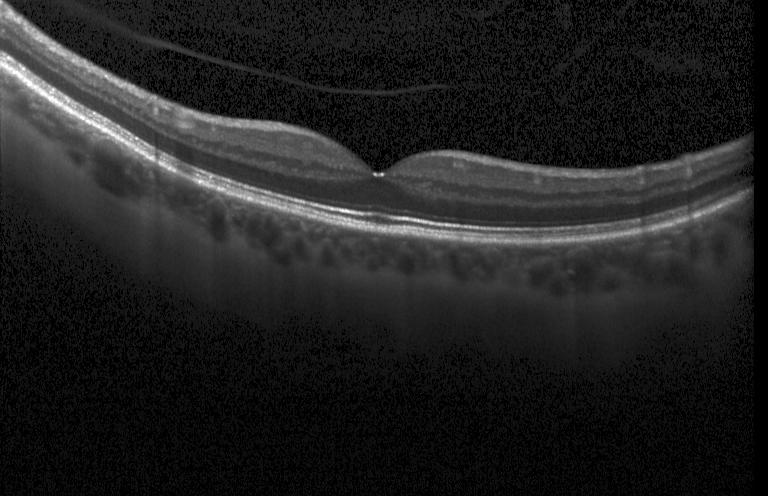
OCT line scan. Acquired on a Heidelberg Spectralis. Impression: no evidence of CNV, DME, or drusen.